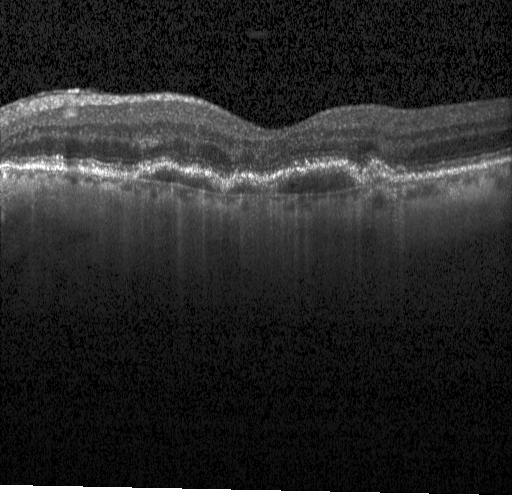
Assessment: choroidal neovascularization (CNV).